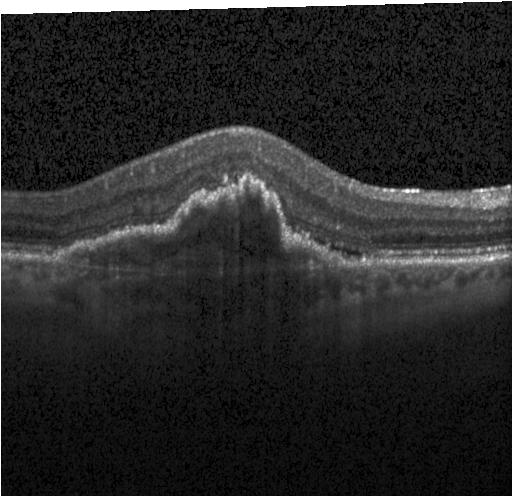
Optical coherence tomography B-scan · horizontal scan through the fovea.
The scan shows a choroidal neovascular membrane.